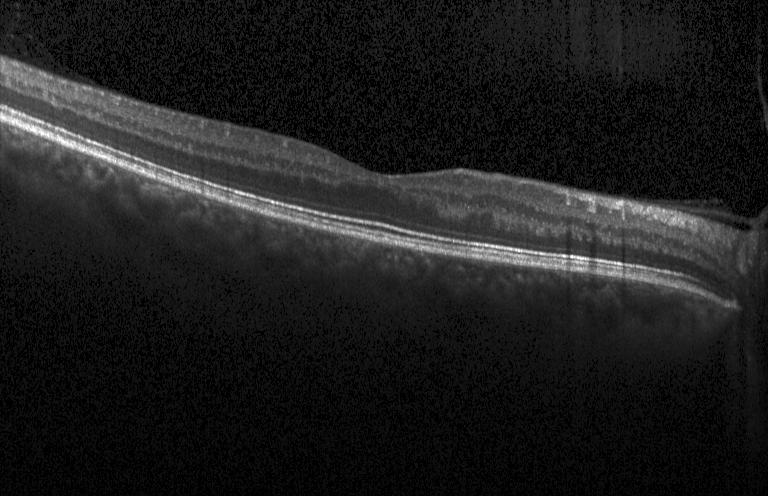

Retinal OCT cross-section
This B-scan demonstrates neither choroidal neovascularization, diabetic macular edema, nor drusen.